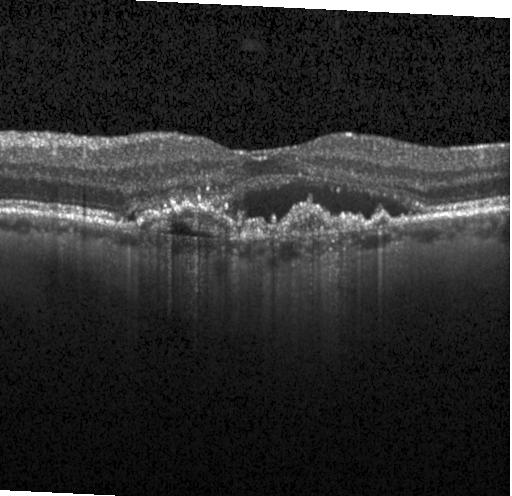

Spectral-domain OCT. Fovea-centered. Instrument: Heidelberg Spectralis. Optical coherence tomography B-scan.
Dx: a choroidal neovascular membrane.